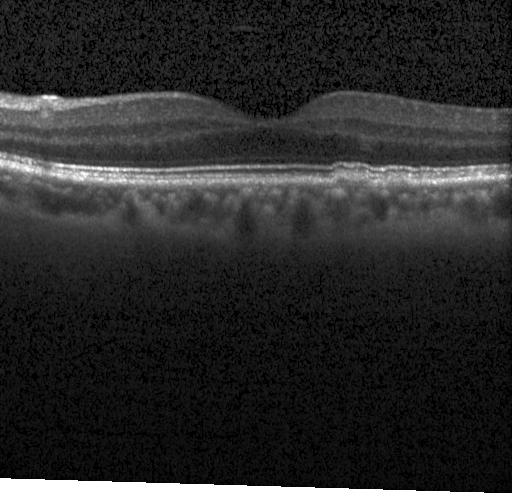
Spectral-domain OCT, OCT B-scan
Finding: sub-RPE drusenoid deposits.